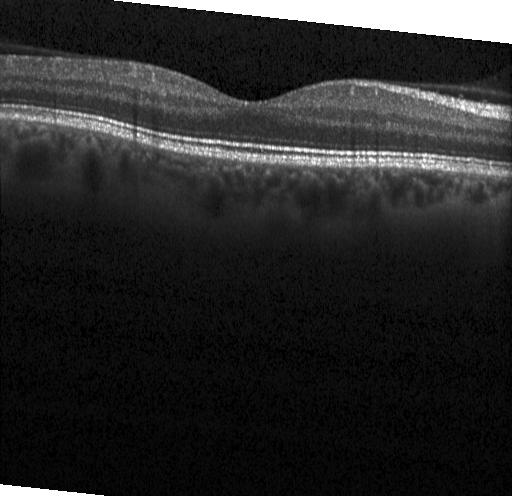
OCT line scan. Centered on the fovea. Acquired on a Heidelberg Spectralis. Finding: no choroidal neovascularization, diabetic macular edema, or drusen.